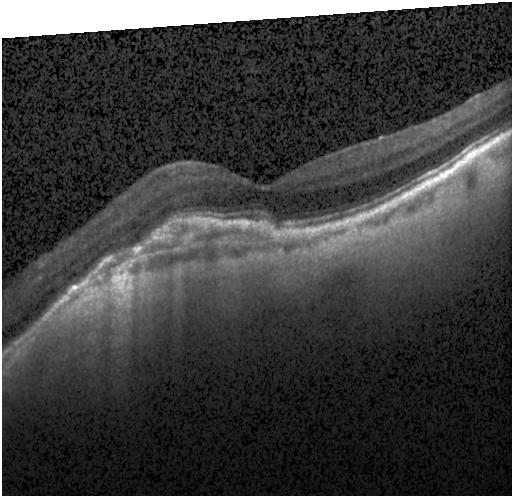 Spectral-domain OCT · retinal OCT cross-section · Heidelberg Spectralis · through the macula.
Assessment: choroidal neovascularization.